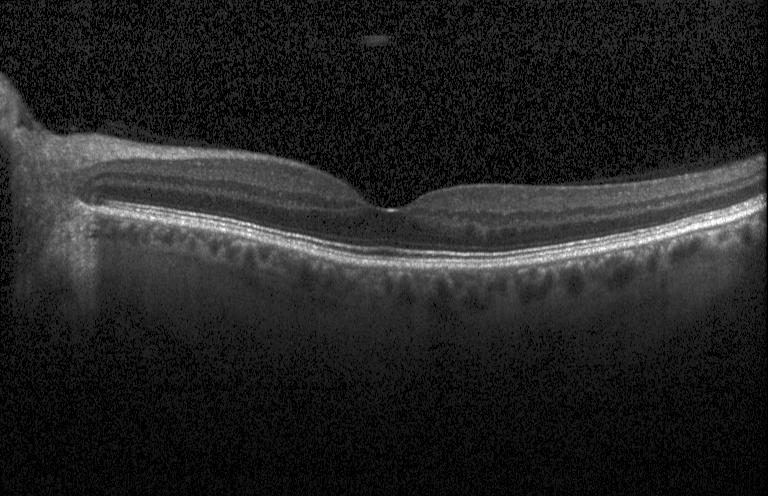
No CNV, no DME, and no drusen.